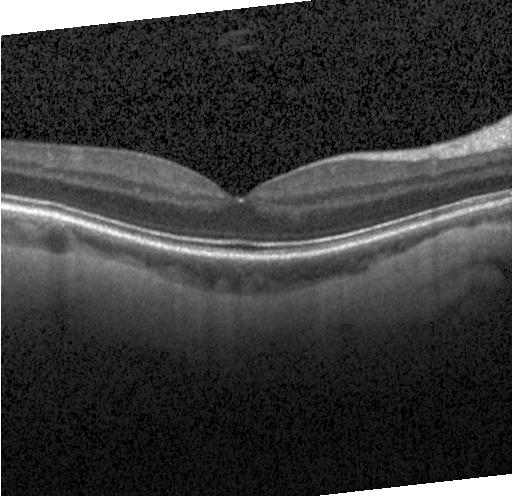
OCT line scan; acquired on a Heidelberg Spectralis — Neither choroidal neovascularization, diabetic macular edema, nor drusen.